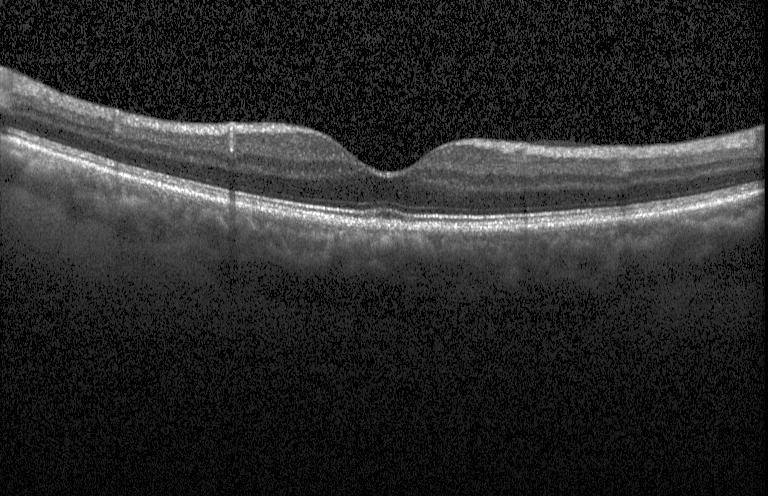 Macular OCT: no evidence of CNV, DME, or drusen.